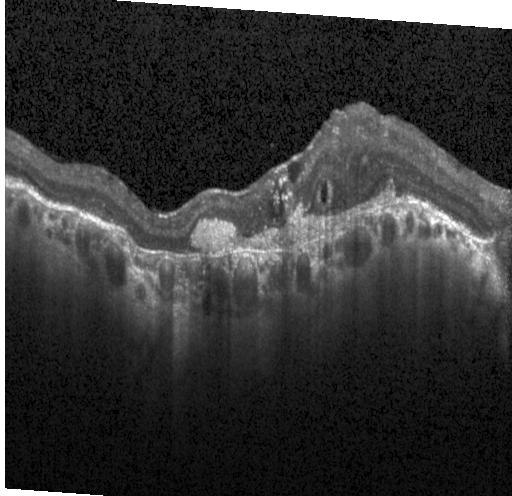

Impression: choroidal neovascularization.